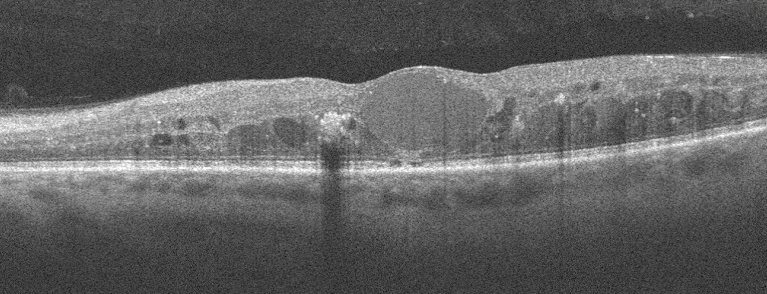

Optical coherence tomography B-scan. Fovea-centered. Acquired on an Optovue Avanti RTVue XR.
Diagnosis: diabetic macular edema.